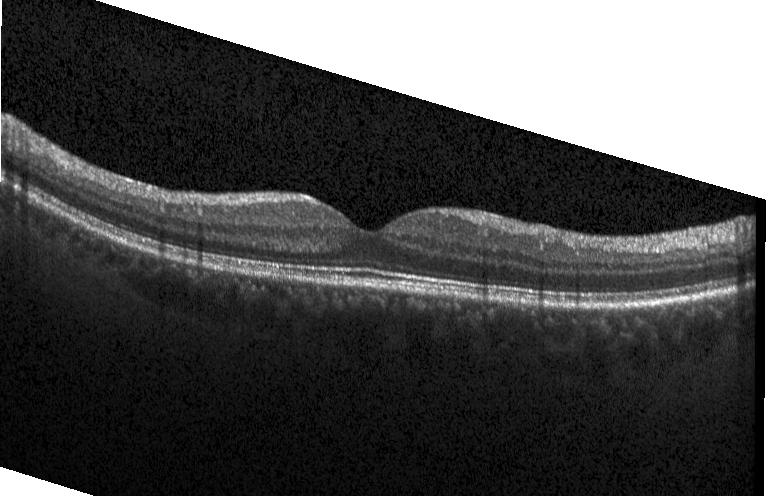
Finding: no CNV, DME, or drusen.